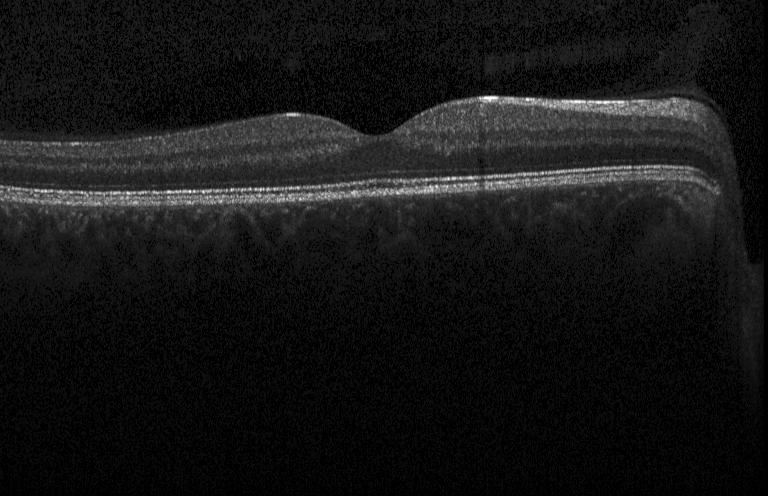

OCT finding: neither CNV, DME, nor drusen.